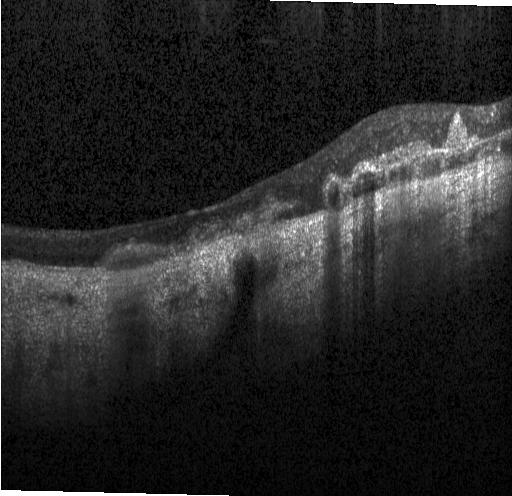 Retinal OCT cross-section
Assessment: a choroidal neovascular membrane.